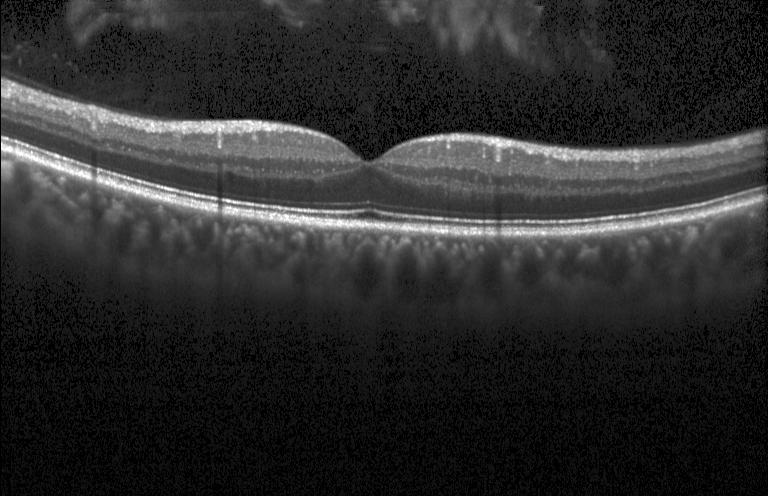 Horizontal scan through the fovea; OCT line scan — OCT finding: no choroidal neovascularization, diabetic macular edema, or drusen.